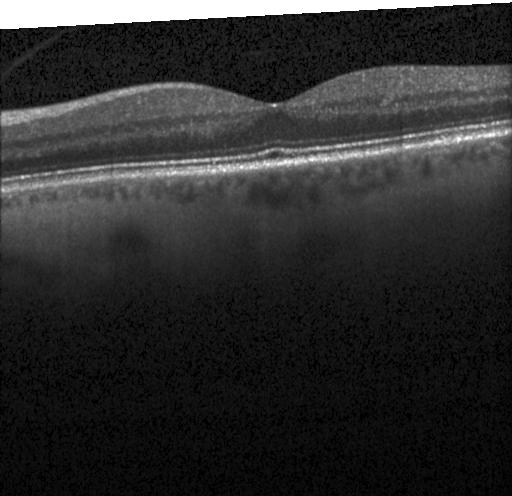

SD-OCT; retinal OCT B-scan. Finding: no choroidal neovascularization, diabetic macular edema, or drusen.